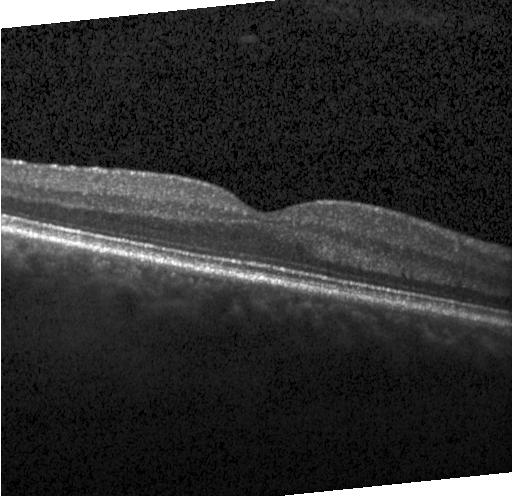 Spectral-domain OCT B-scan: no choroidal neovascularization, no diabetic macular edema, and no drusen.